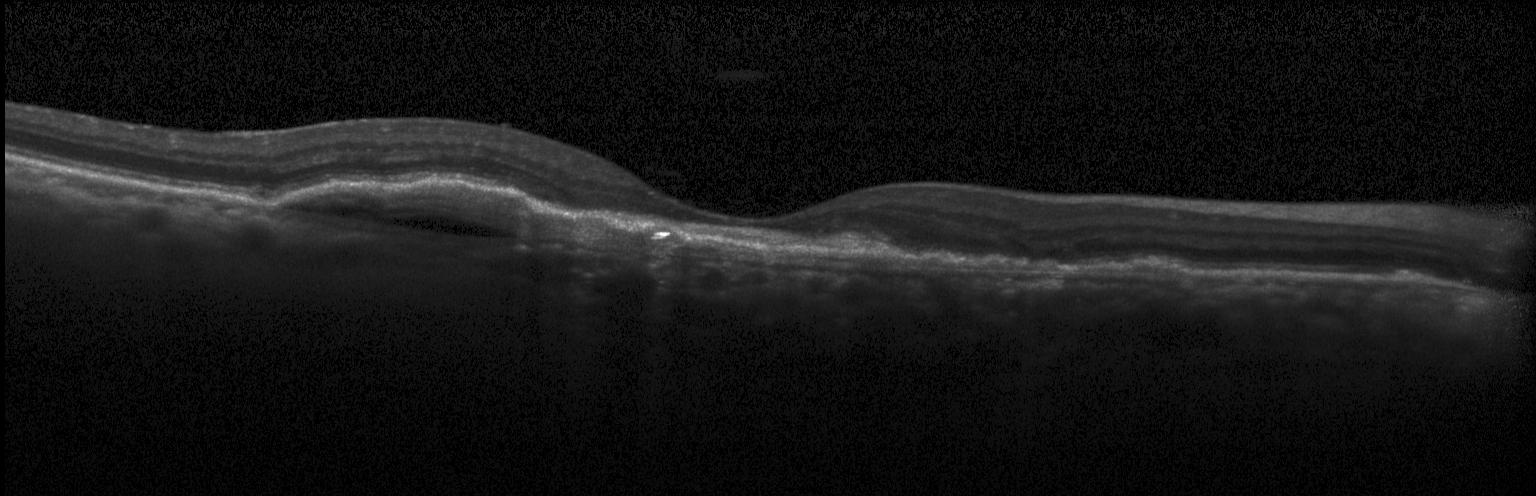

Macular scan · OCT line scan
Assessment: a choroidal neovascular membrane.